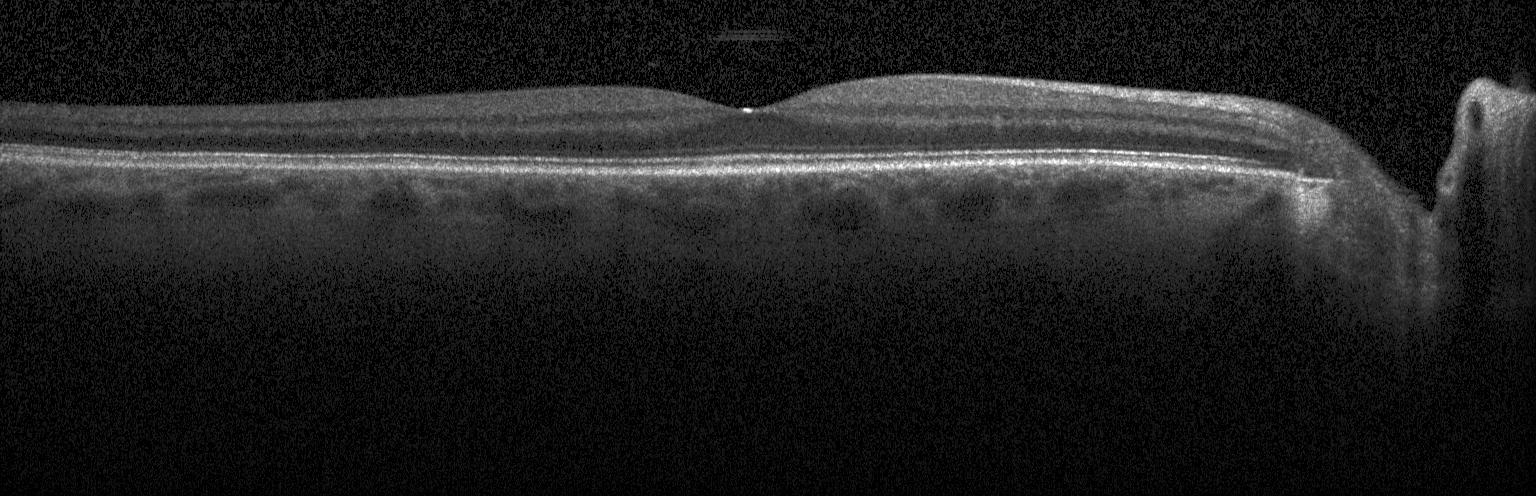
Macular OCT: no evidence of choroidal neovascularization, diabetic macular edema, or drusen.